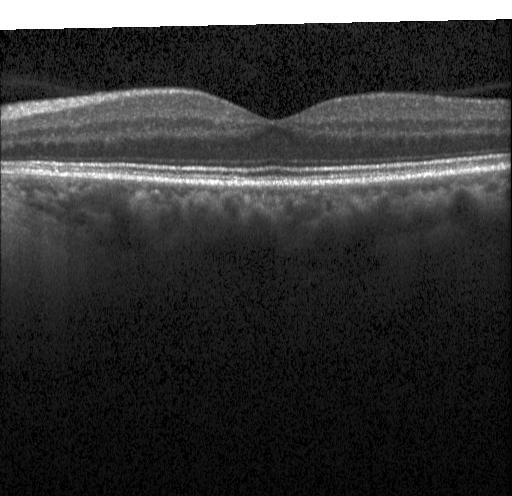 OCT B-scan, macular scan. Finding: no choroidal neovascularization, no diabetic macular edema, and no drusen.